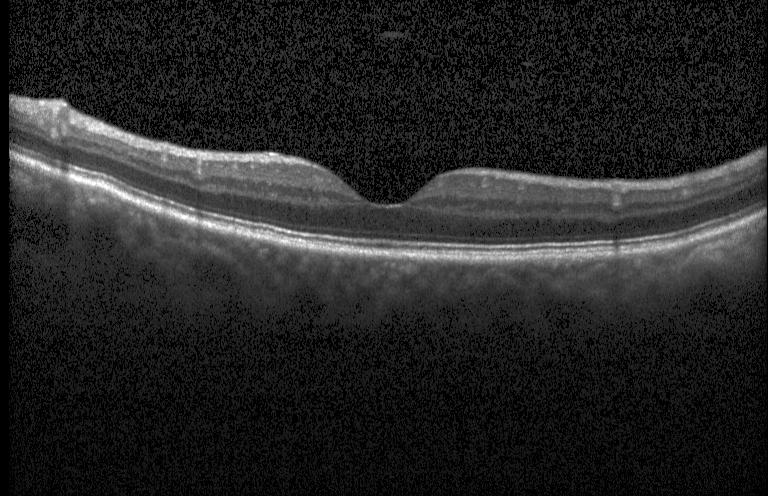
Heidelberg Spectralis OCT system, OCT line scan.
Finding: no CNV, no DME, and no drusen.